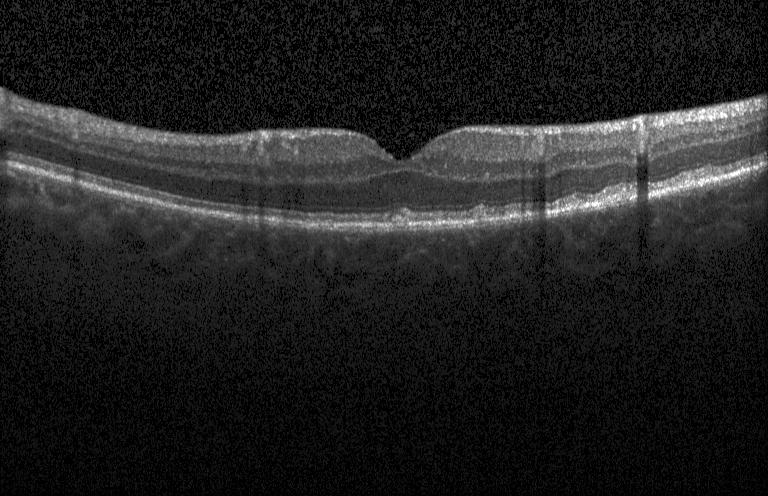 Spectral-domain OCT, optical coherence tomography B-scan, macular scan, Heidelberg Spectralis. Impression: drusen.